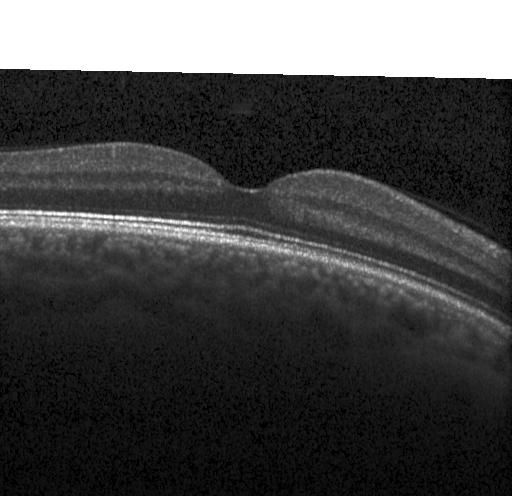 OCT B-scan, macular scan, Heidelberg Spectralis — Diagnosis: no CNV, no DME, and no drusen.